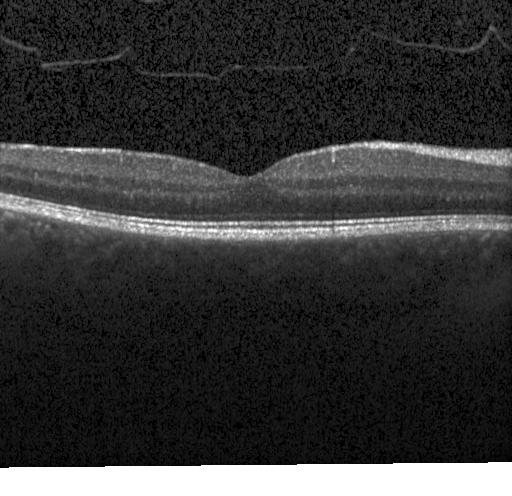 OCT line scan.
Finding: no choroidal neovascularization, no diabetic macular edema, and no drusen.